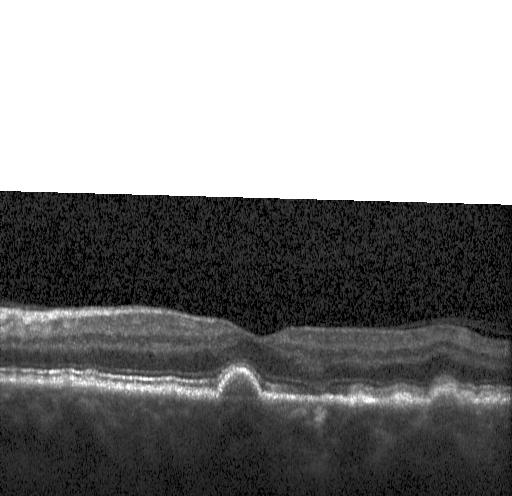

Diagnosis: multiple drusen.